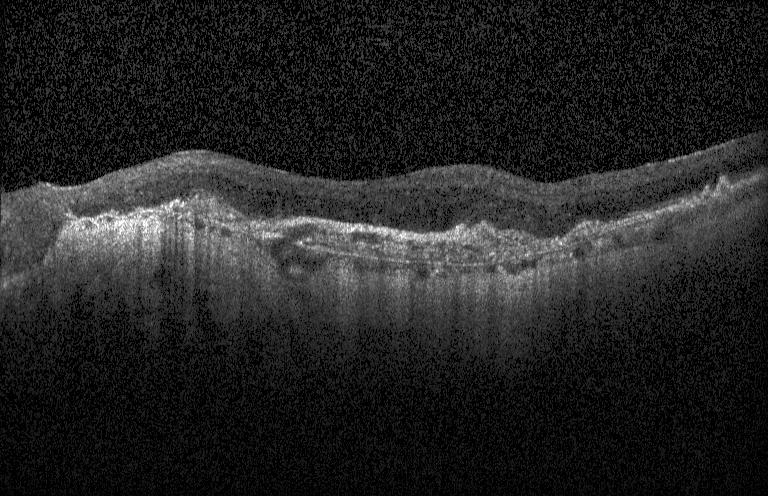
Fovea-centered. Spectral-domain OCT. Retinal OCT B-scan. Heidelberg Spectralis.
This B-scan demonstrates choroidal neovascularization.